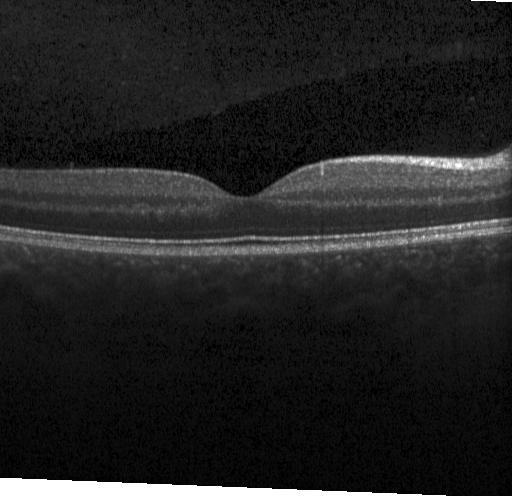

Diagnosis: no evidence of choroidal neovascularization, diabetic macular edema, or drusen.